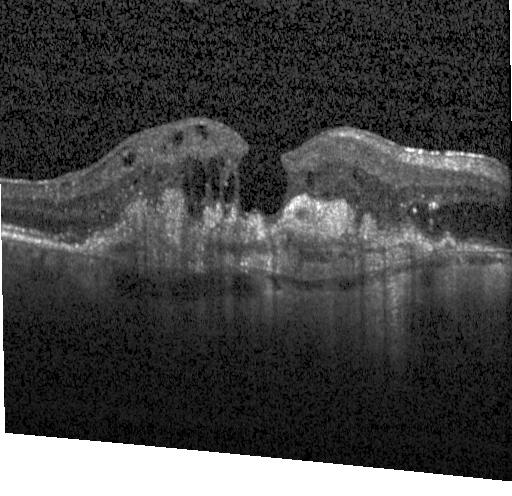 Finding: choroidal neovascularization.